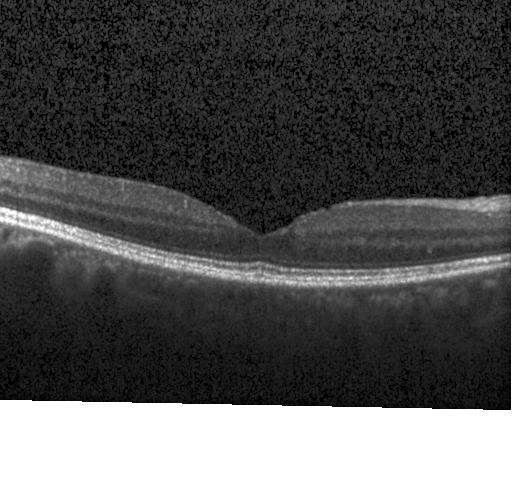
This B-scan demonstrates neither choroidal neovascularization, diabetic macular edema, nor drusen.